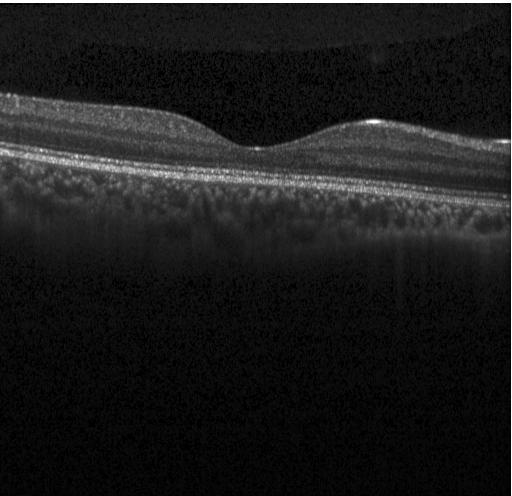

Spectral-domain optical coherence tomography · Heidelberg Spectralis OCT system · optical coherence tomography scan.
No evidence of choroidal neovascularization, diabetic macular edema, or drusen.